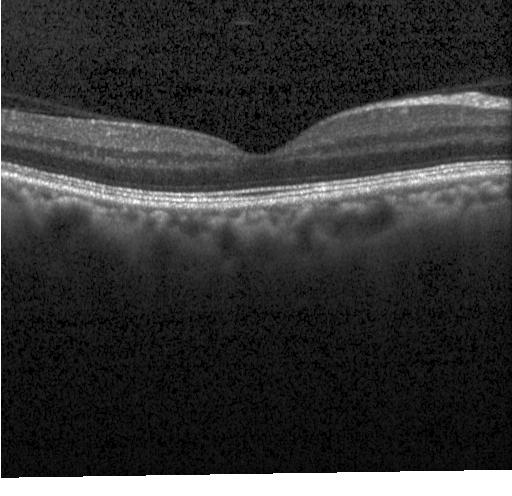

OCT finding: neither CNV, DME, nor drusen.